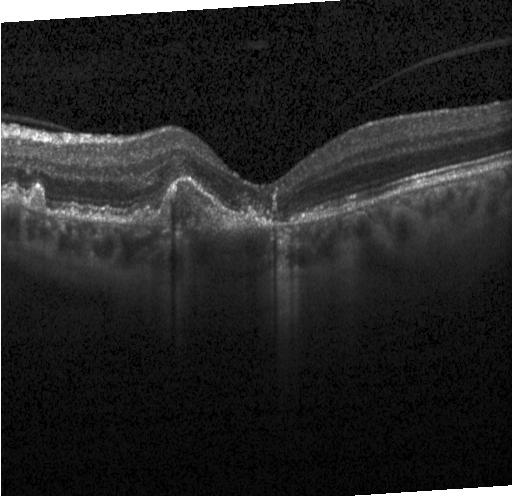
Spectral-domain OCT. Retinal OCT cross-section
Impression: choroidal neovascularization.